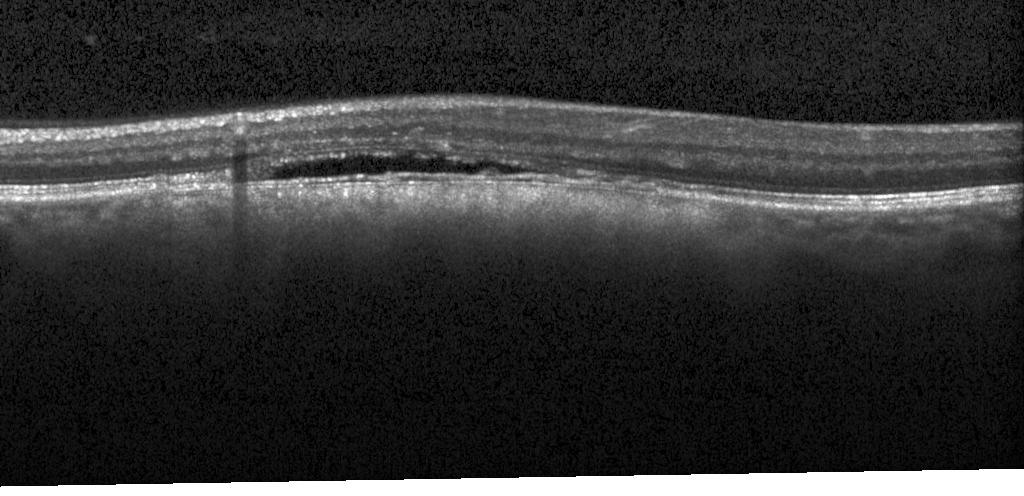

This B-scan demonstrates CNV.